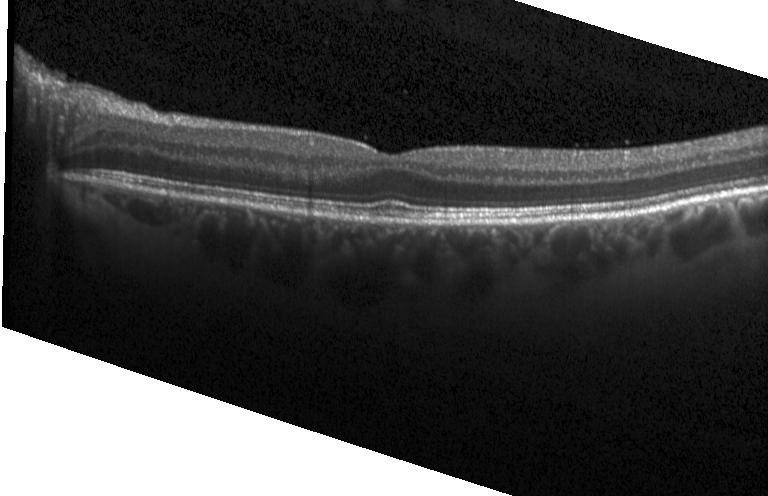
This B-scan demonstrates neither choroidal neovascularization, diabetic macular edema, nor drusen.